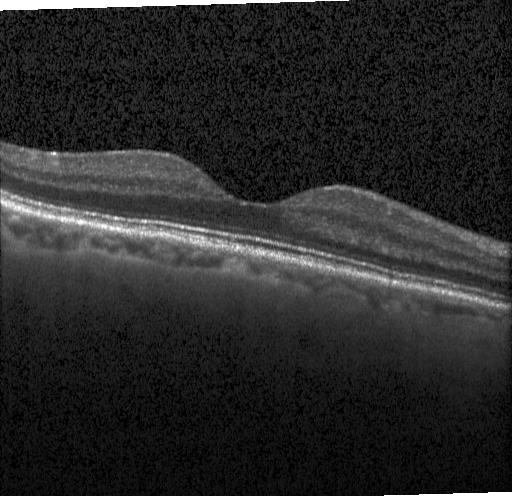

Impression: neither choroidal neovascularization, diabetic macular edema, nor drusen.